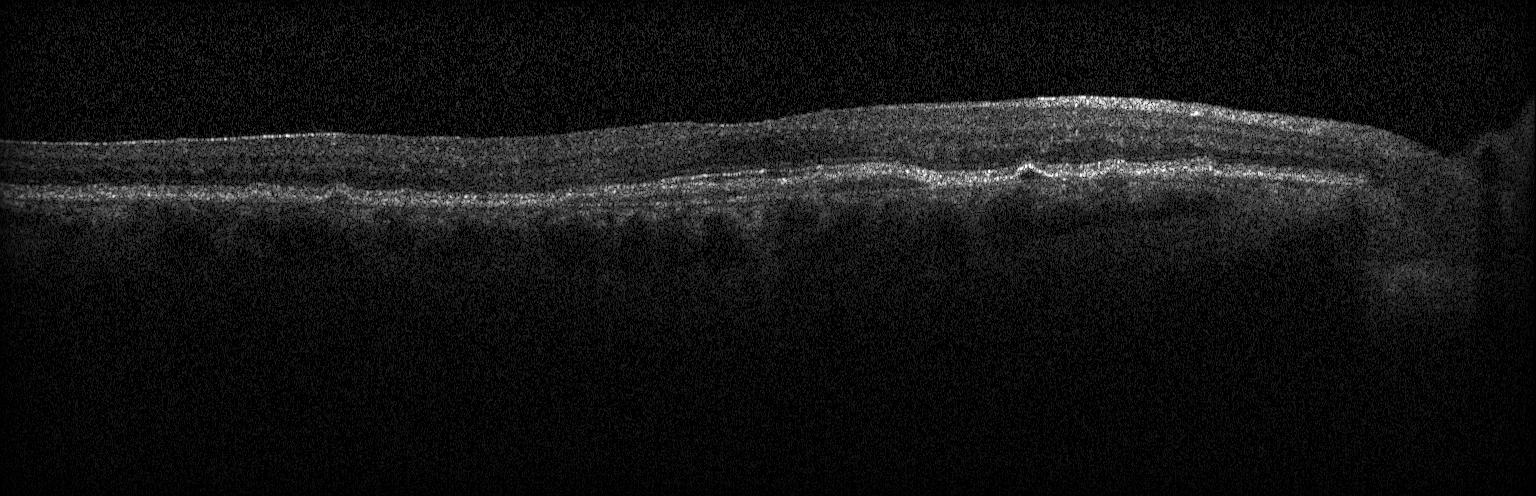

Diagnosis: a choroidal neovascular membrane.